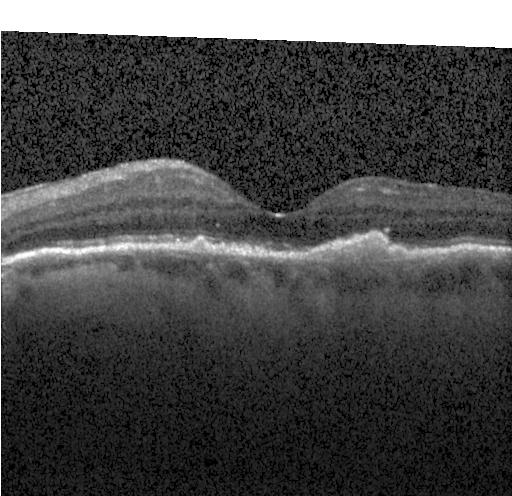 The scan shows choroidal neovascularization.